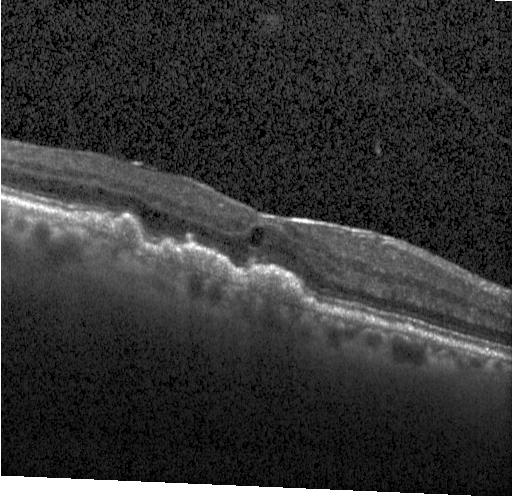 Macular OCT demonstrating a choroidal neovascular membrane.